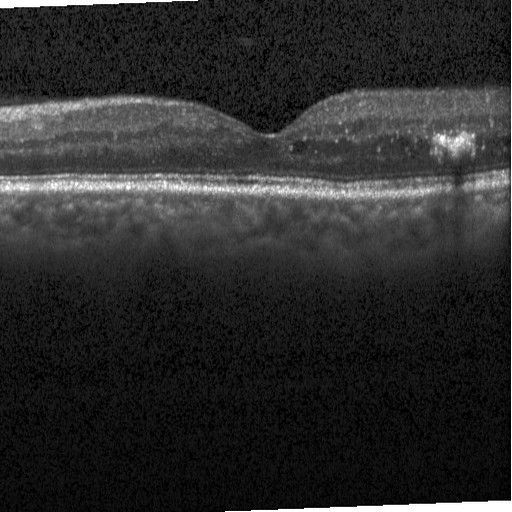

Optical coherence tomography scan.
Diabetic macular edema (DME).